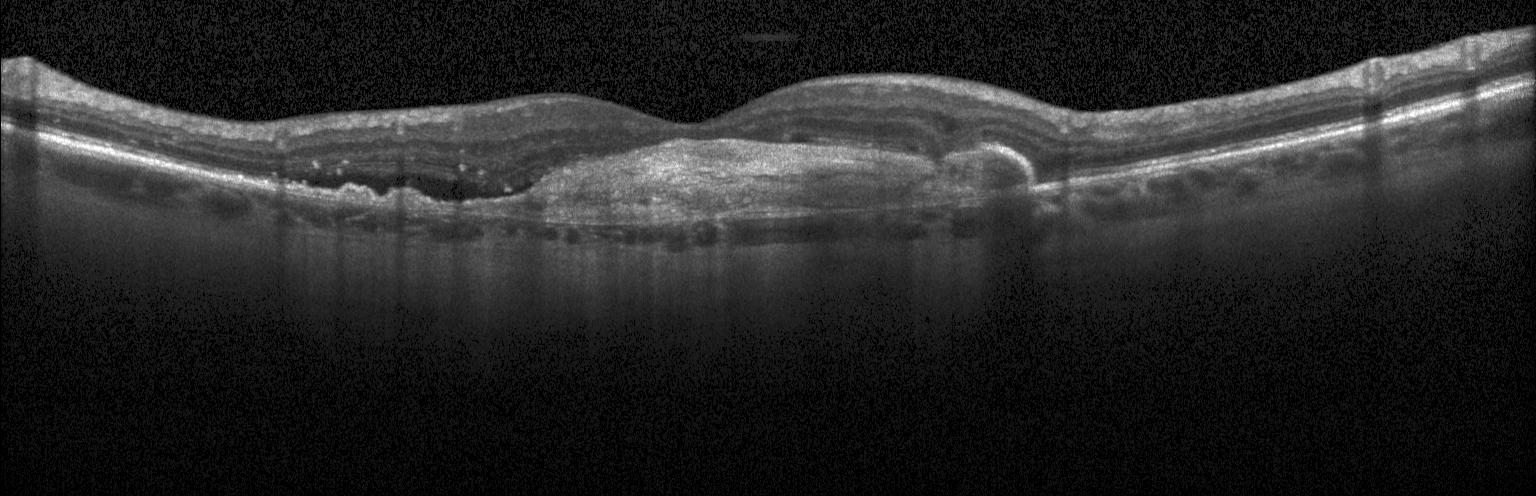
Spectral-domain OCT; OCT B-scan.
Diagnosis: a choroidal neovascular membrane.